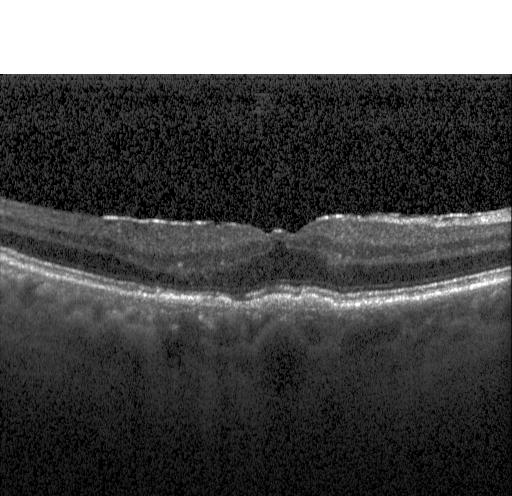
Horizontal scan through the fovea, instrument: Heidelberg Spectralis, SD-OCT, optical coherence tomography scan
This B-scan demonstrates choroidal neovascularization.